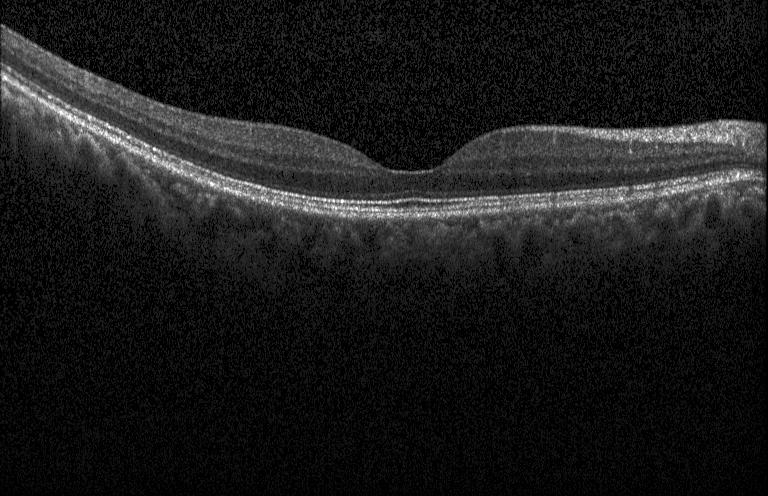

Optical coherence tomography scan. Finding: no CNV, no DME, and no drusen.